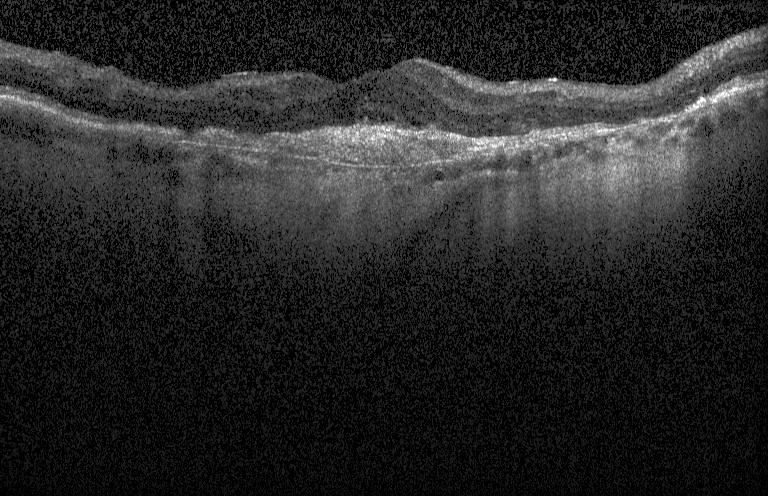
Macular OCT demonstrating choroidal neovascularization (CNV).